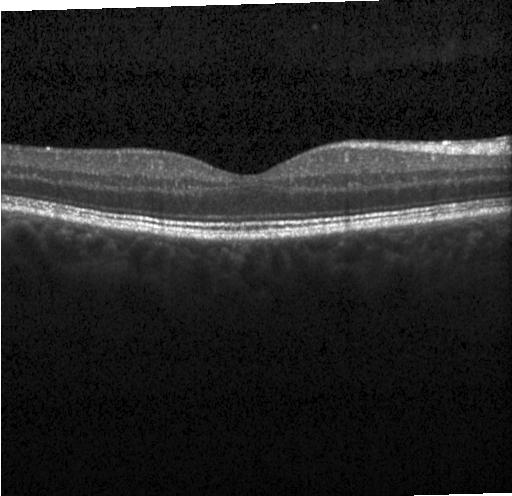 Impression: no choroidal neovascularization, diabetic macular edema, or drusen.